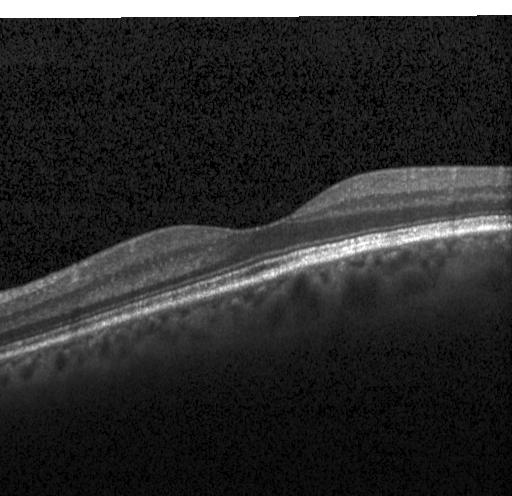 Diagnosis: no choroidal neovascularization, no diabetic macular edema, and no drusen.